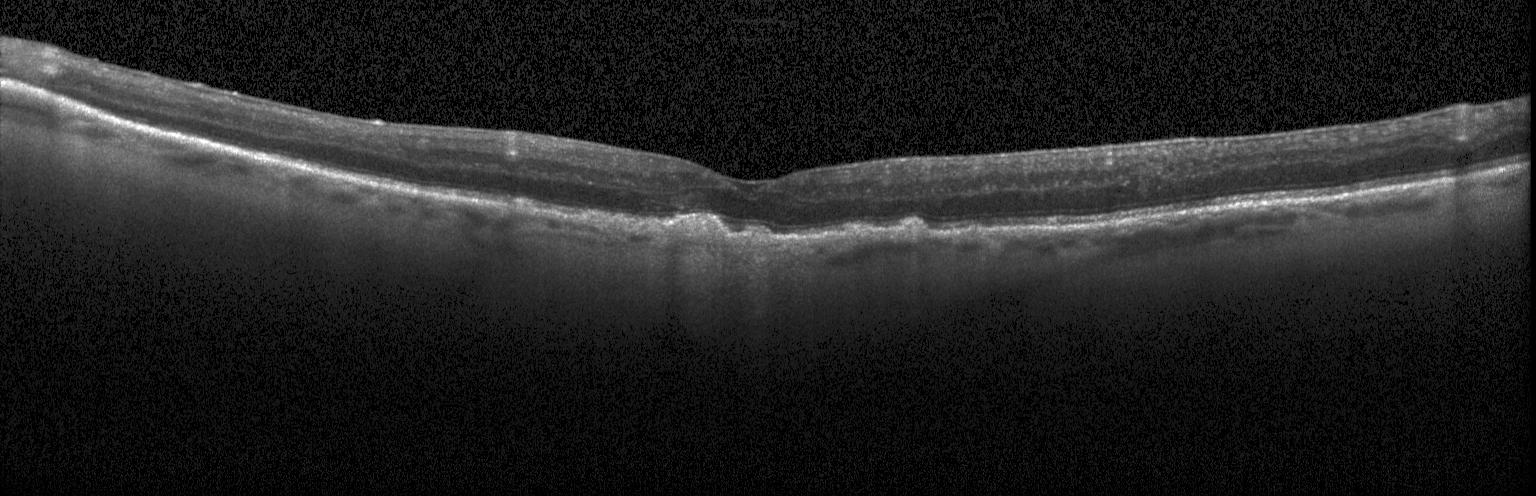
Retinal OCT cross-section; SD-OCT
Choroidal neovascularization (CNV).